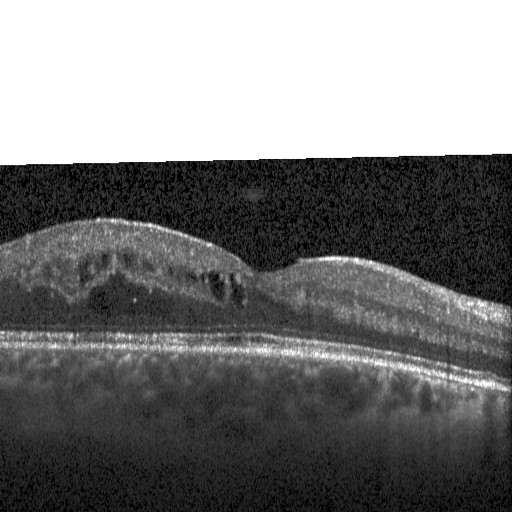
Retinal OCT B-scan. Acquired on a Heidelberg Spectralis. Spectral-domain OCT — Diagnosis: diabetic macular edema (DME).